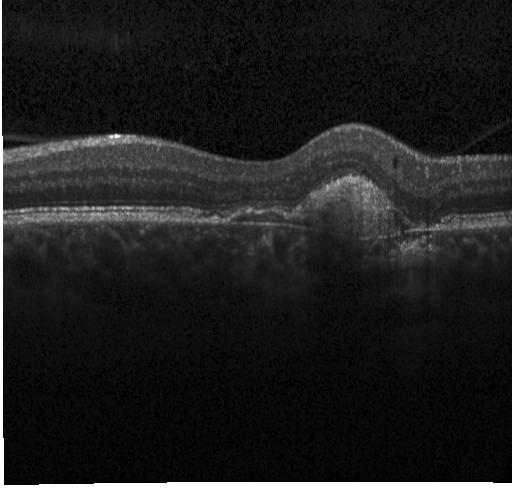

SD-OCT · fovea-centered · retinal OCT cross-section · instrument: Heidelberg Spectralis.
CNV.